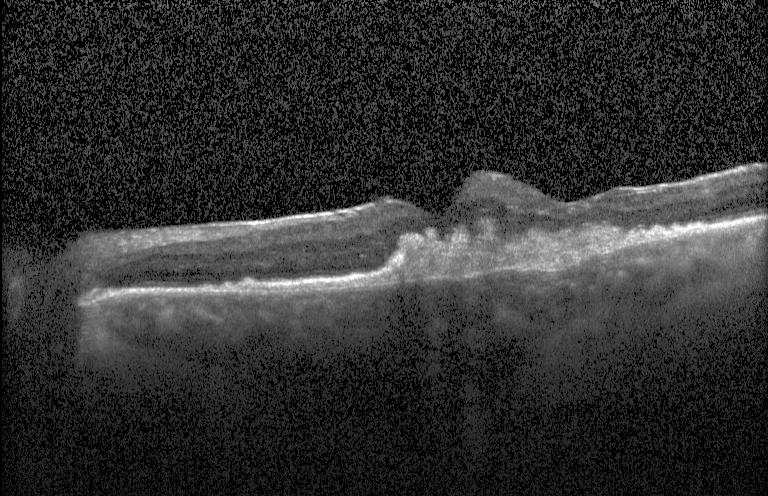 Choroidal neovascularization.